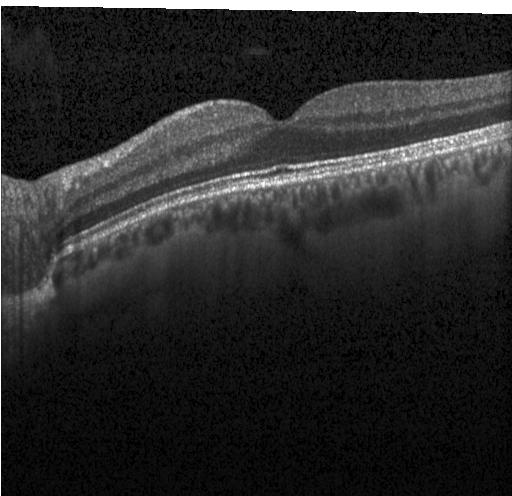
Macular scan, Heidelberg Spectralis, OCT B-scan, spectral-domain optical coherence tomography.
Finding: no CNV, DME, or drusen.